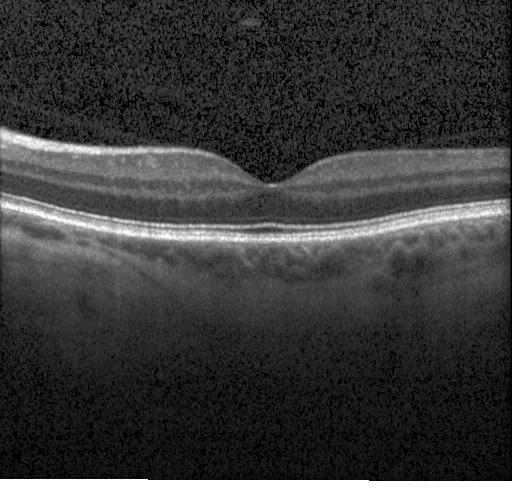

Dx: no CNV, no DME, and no drusen.